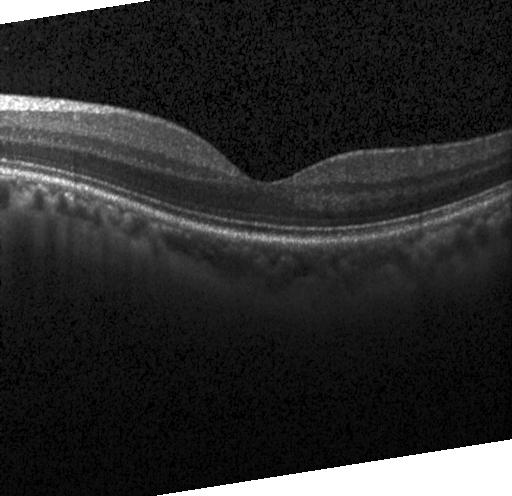 Retinal OCT B-scan.
Finding: no choroidal neovascularization, no diabetic macular edema, and no drusen.